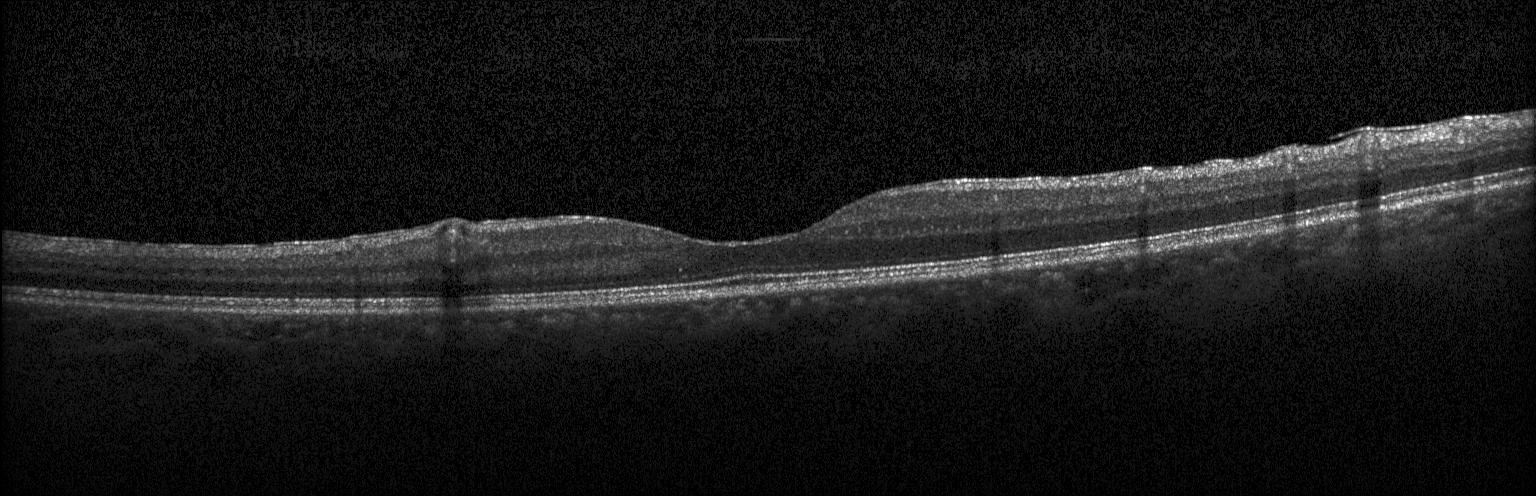
Finding: neither CNV, DME, nor drusen.